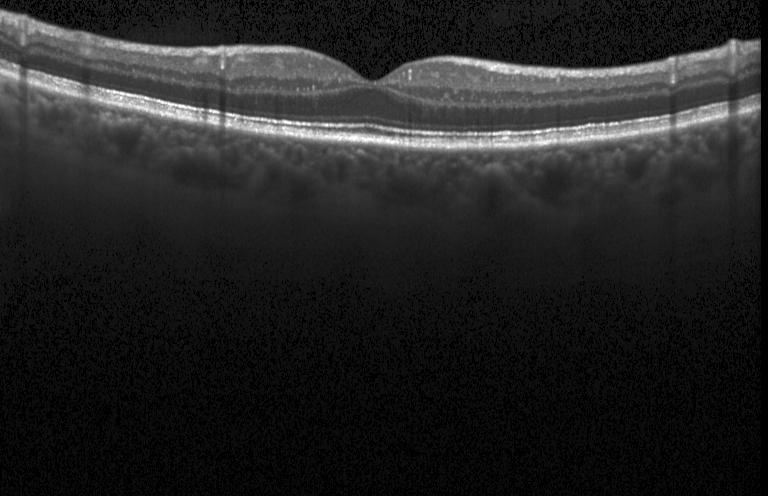

Retinal OCT cross-section.
Dx: no CNV, no DME, and no drusen.